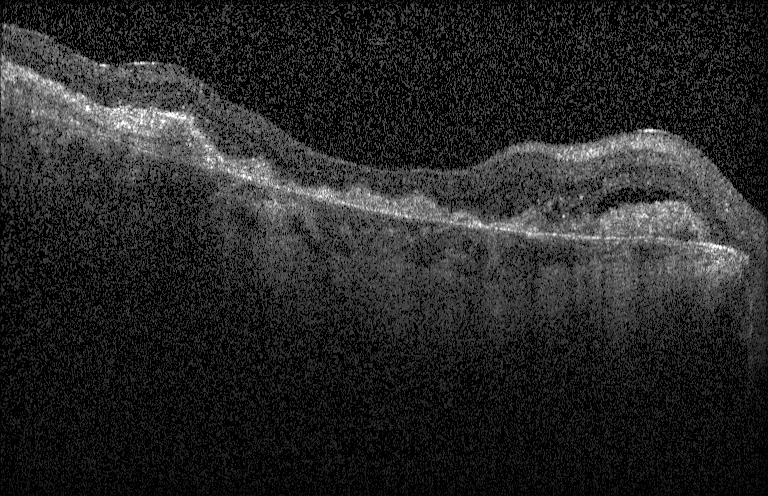
Through the macula. Acquired on a Heidelberg Spectralis. Spectral-domain OCT. Optical coherence tomography B-scan
Macular OCT: a choroidal neovascular membrane.